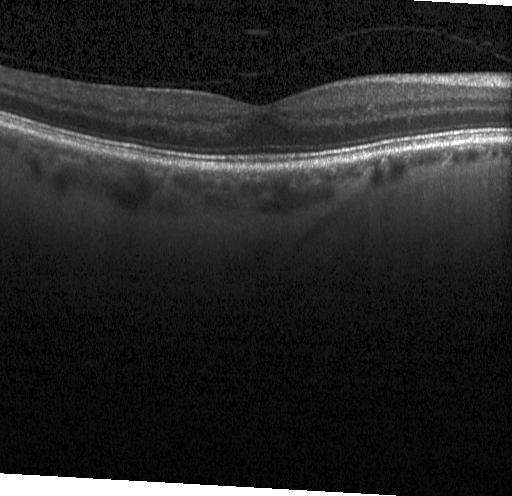

OCT finding: no choroidal neovascularization, diabetic macular edema, or drusen.